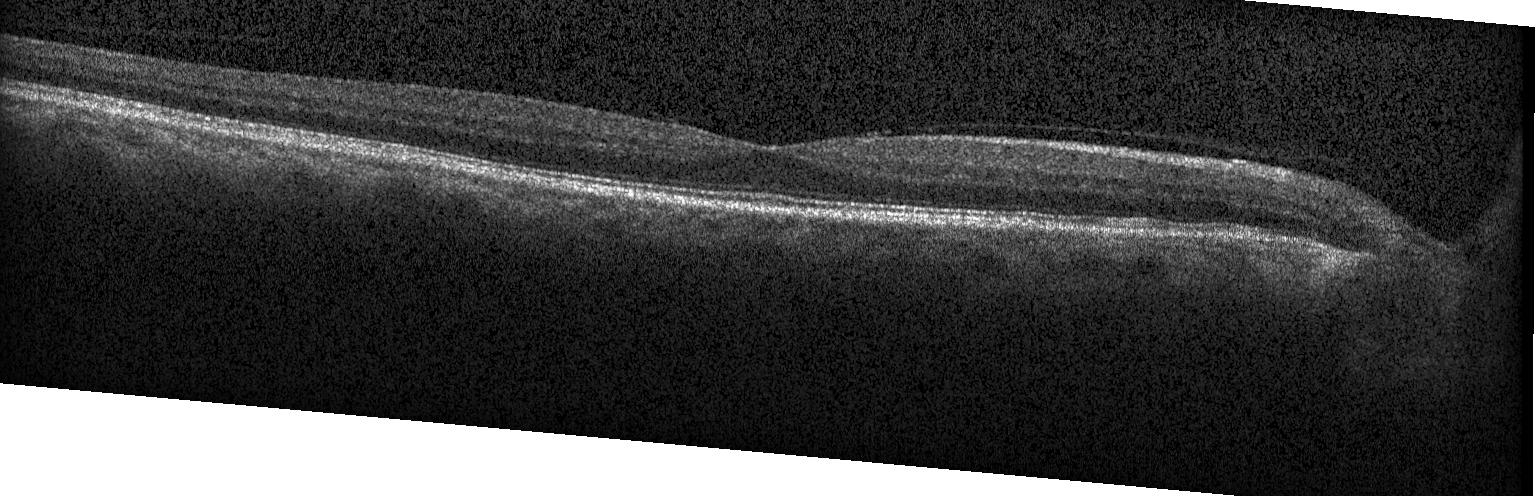 Horizontal scan through the fovea, retinal OCT cross-section, spectral-domain optical coherence tomography — Impression: no evidence of CNV, DME, or drusen.